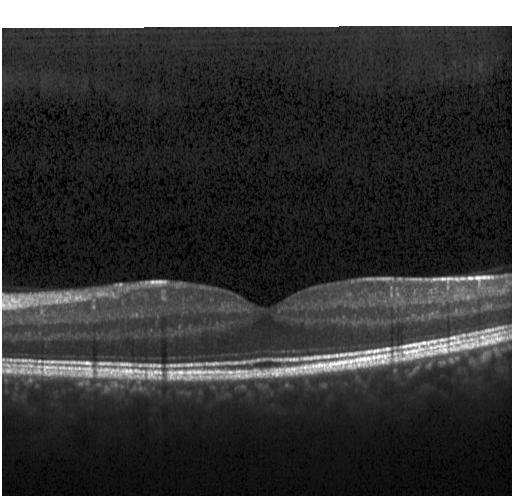 Retinal OCT cross-section showing no CNV, no DME, and no drusen.